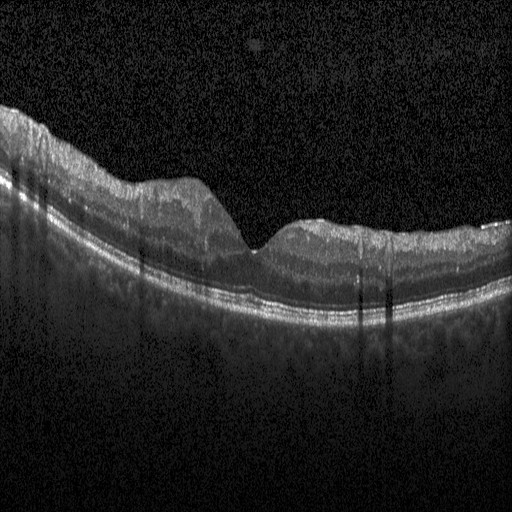 Retinal OCT B-scan — The scan shows diabetic macular edema.